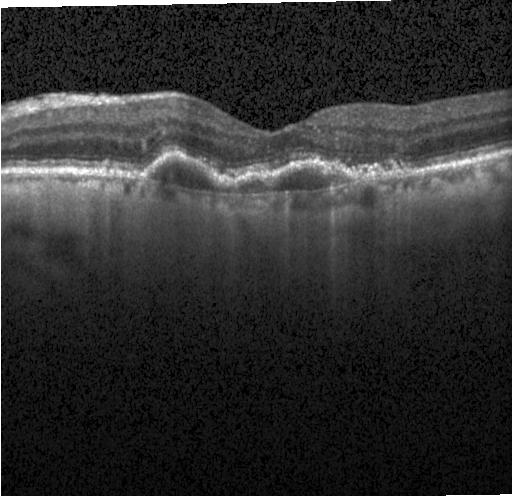

Spectral-domain optical coherence tomography · retinal OCT cross-section · Heidelberg Spectralis
Impression: a choroidal neovascular membrane.